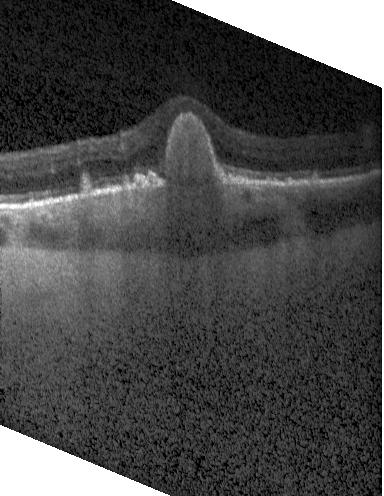
Finding: a choroidal neovascular membrane.